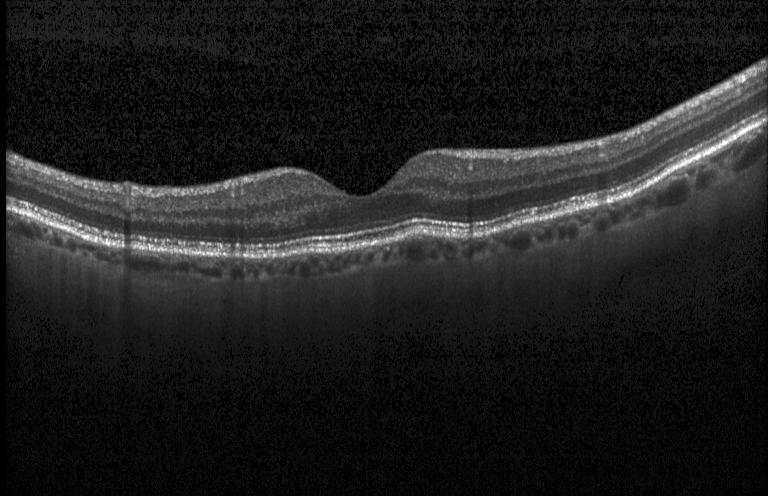 No choroidal neovascularization, no diabetic macular edema, and no drusen.